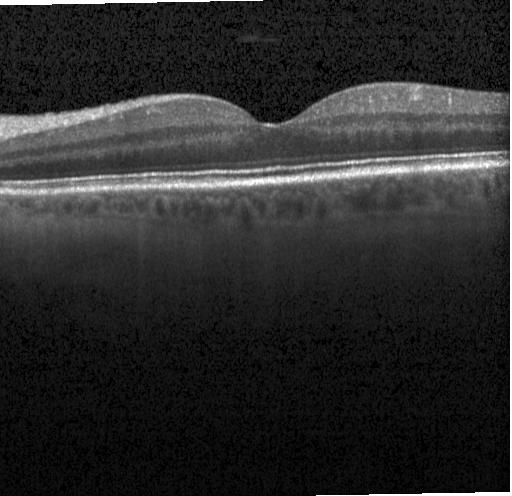 Optical coherence tomography B-scan. Heidelberg Spectralis.
Diagnosis: no evidence of CNV, DME, or drusen.